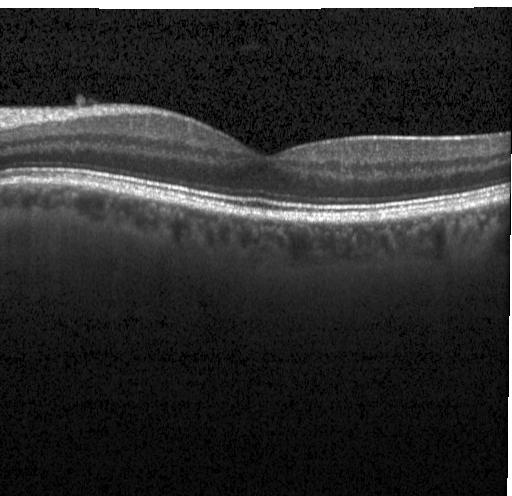 Finding: no choroidal neovascularization, diabetic macular edema, or drusen.